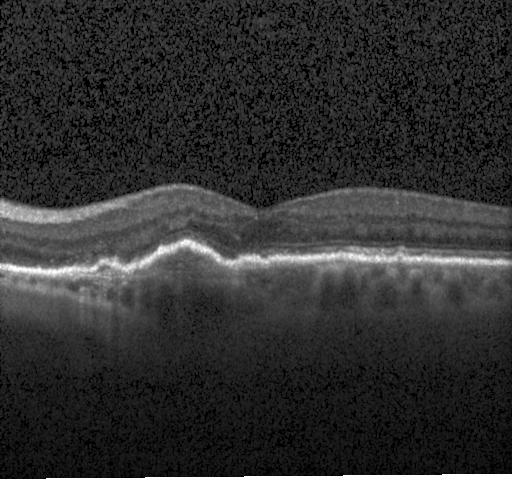 Diagnosis: a choroidal neovascular membrane.